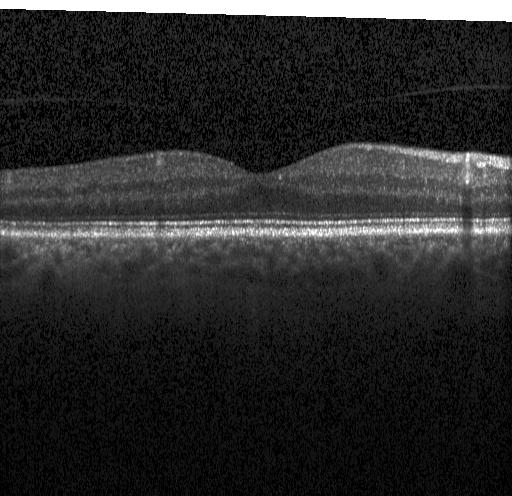 Retinal OCT cross-section — Finding: no choroidal neovascularization, diabetic macular edema, or drusen.